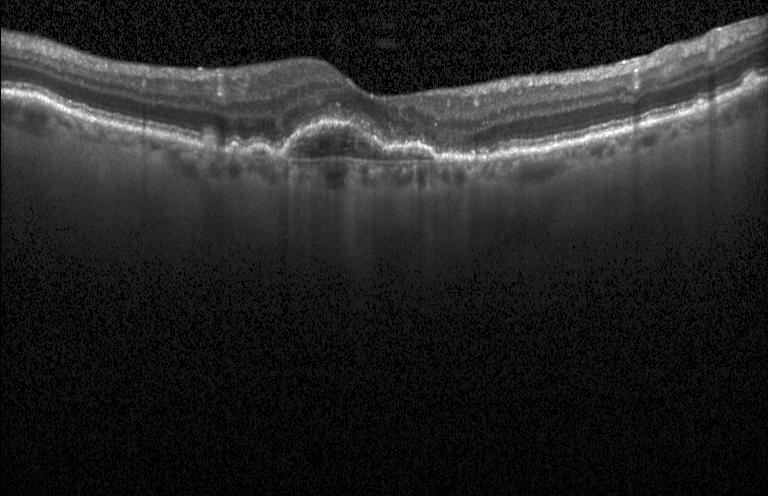

Impression: choroidal neovascularization (CNV).